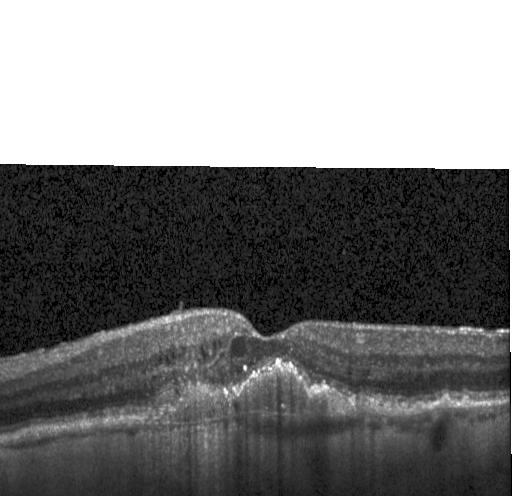
Retinal OCT B-scan; macular scan.
OCT finding: a choroidal neovascular membrane.